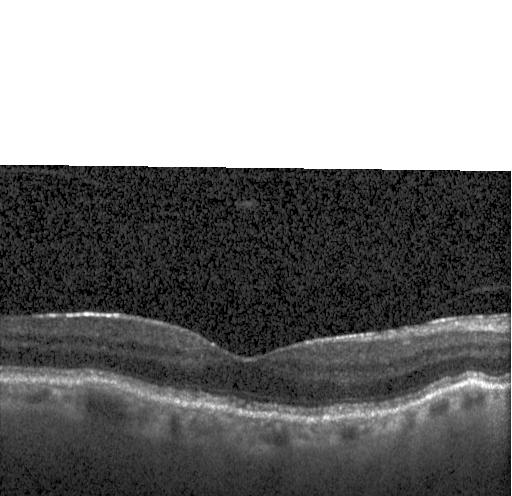

OCT line scan · centered on the fovea · spectral-domain OCT. No evidence of choroidal neovascularization, diabetic macular edema, or drusen.